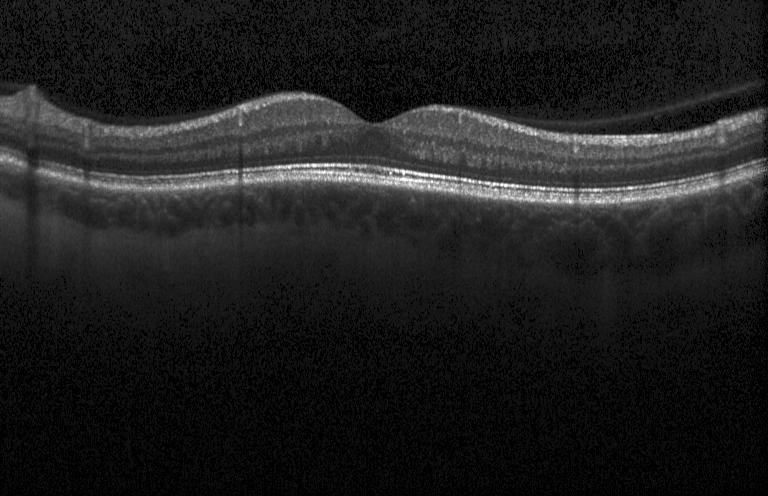
Assessment: neither CNV, DME, nor drusen.